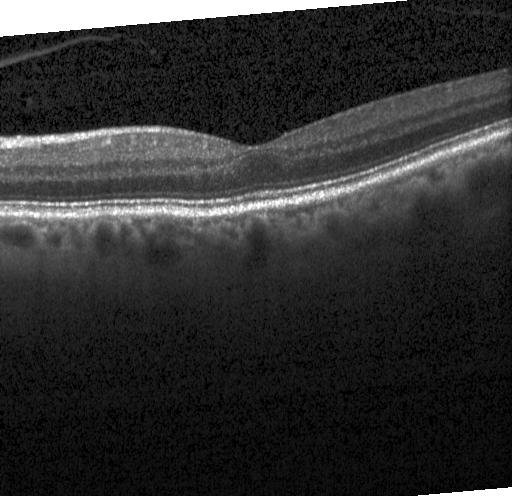
Centered on the fovea, OCT B-scan, acquired on a Heidelberg Spectralis, spectral-domain OCT. Impression: no evidence of choroidal neovascularization, diabetic macular edema, or drusen.